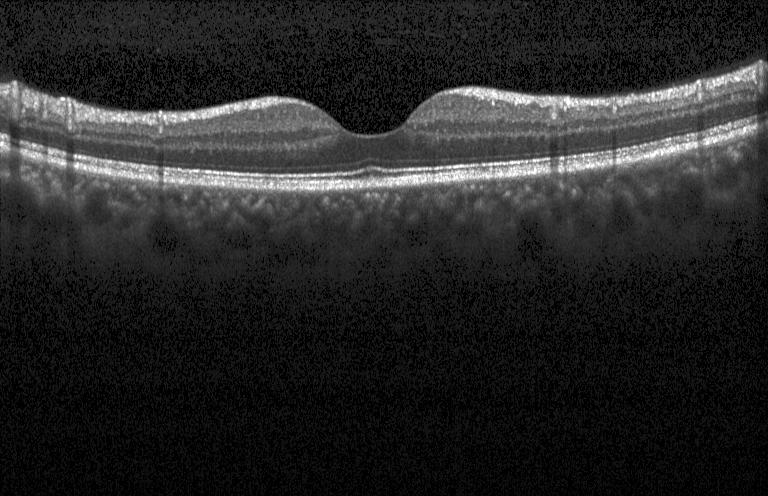
OCT line scan — Finding: no choroidal neovascularization, no diabetic macular edema, and no drusen.